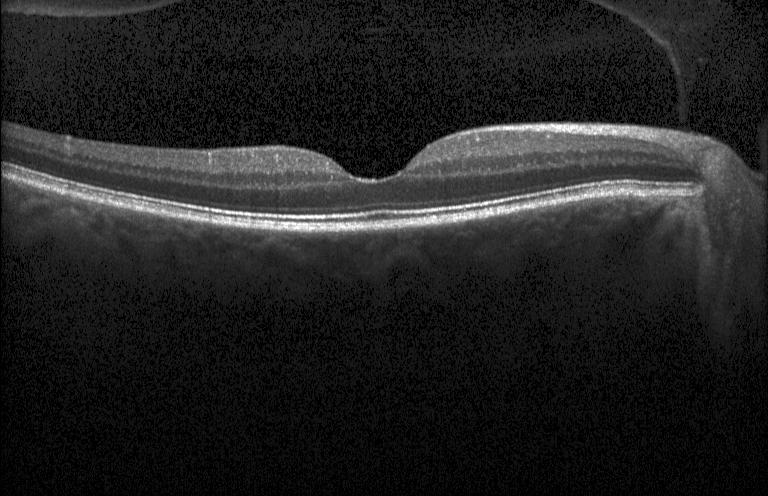

Finding: no evidence of choroidal neovascularization, diabetic macular edema, or drusen.